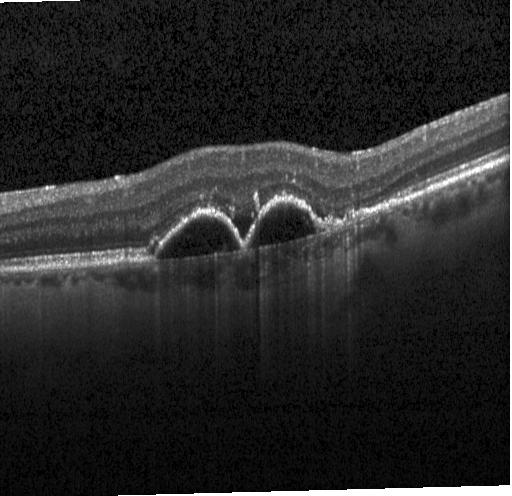
Optical coherence tomography scan. Centered on the fovea. Spectral-domain OCT
Finding: choroidal neovascularization.